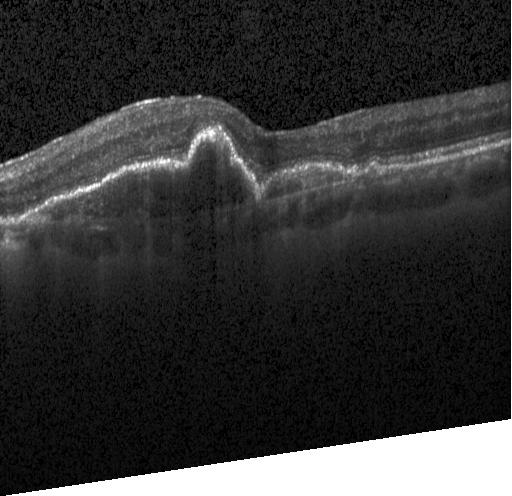 Spectral-domain OCT. Optical coherence tomography B-scan — Dx: a choroidal neovascular membrane.